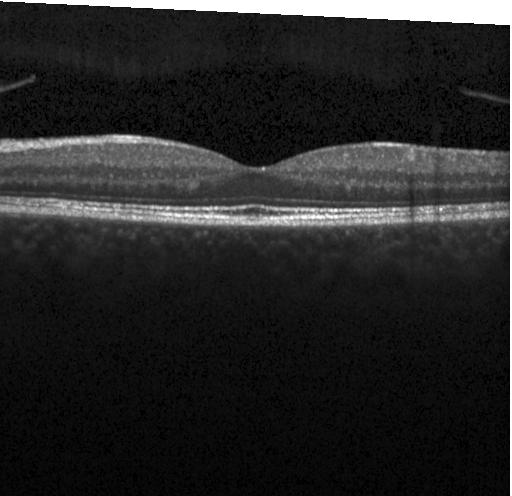

Finding: no evidence of CNV, DME, or drusen.